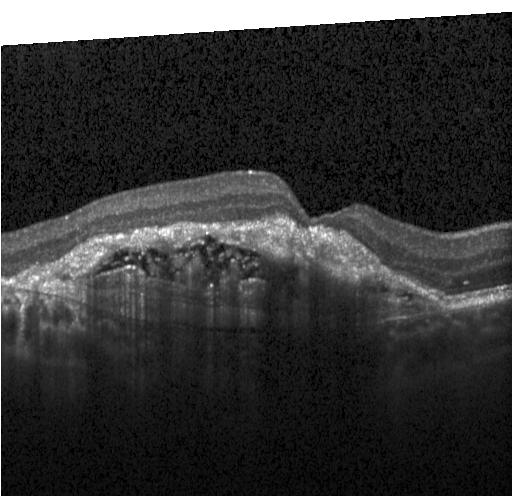

Finding: choroidal neovascularization (CNV).